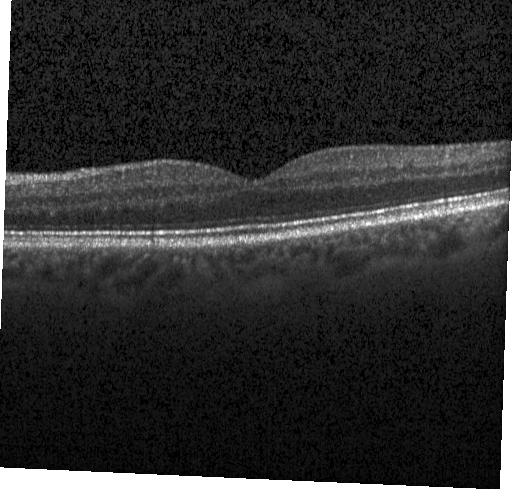 OCT B-scan.
No choroidal neovascularization, diabetic macular edema, or drusen.